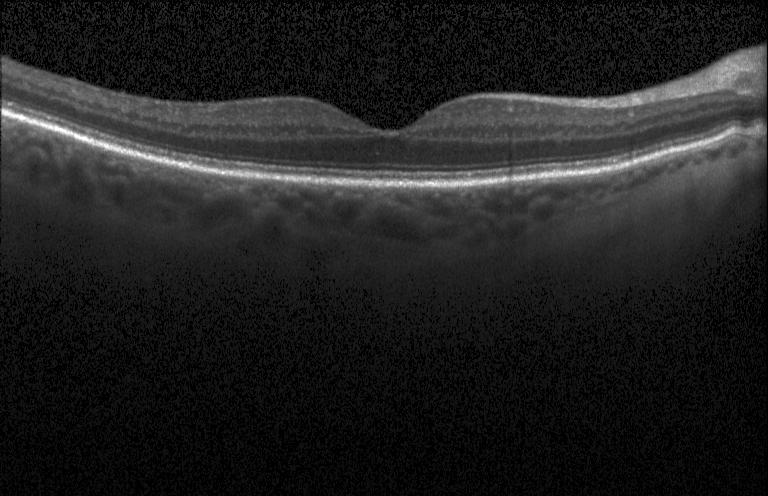 Assessment: neither choroidal neovascularization, diabetic macular edema, nor drusen.